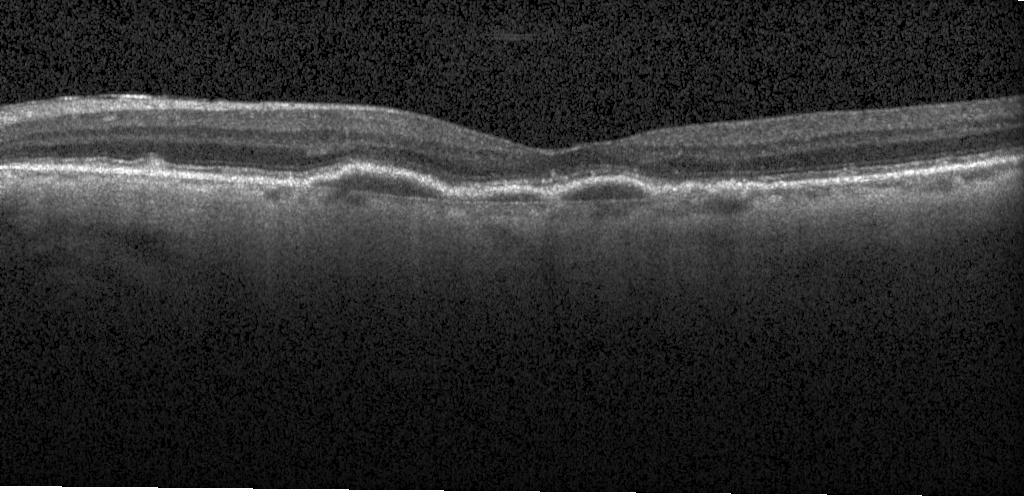
Optical coherence tomography B-scan — This B-scan demonstrates a choroidal neovascular membrane.